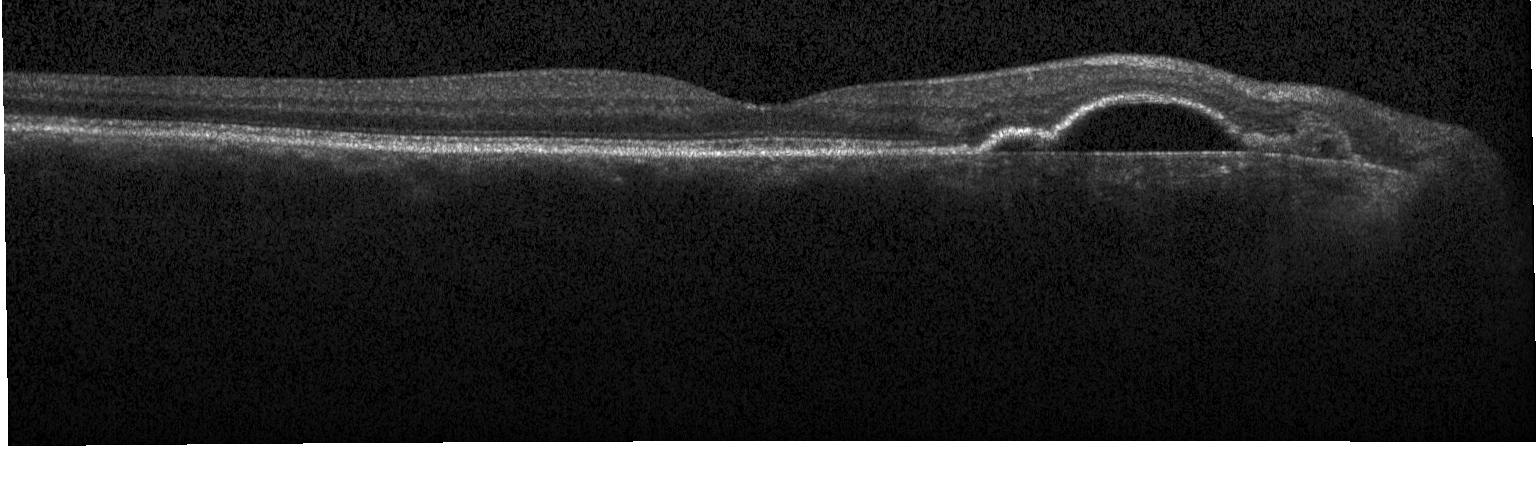

Retinal OCT B-scan, spectral-domain optical coherence tomography, acquired on a Heidelberg Spectralis, centered on the fovea.
The scan shows choroidal neovascularization (CNV).